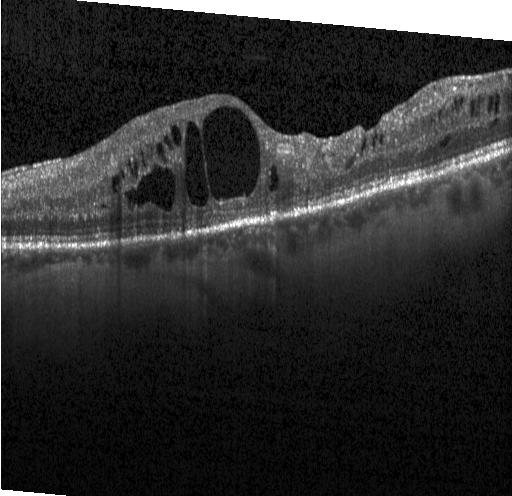 Through the macula; retinal OCT B-scan; spectral-domain OCT; Heidelberg Spectralis. The scan shows diabetic macular edema.